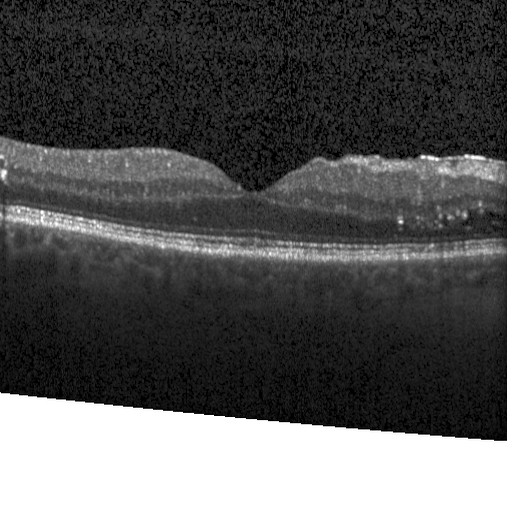

OCT finding: diabetic macular edema (DME).